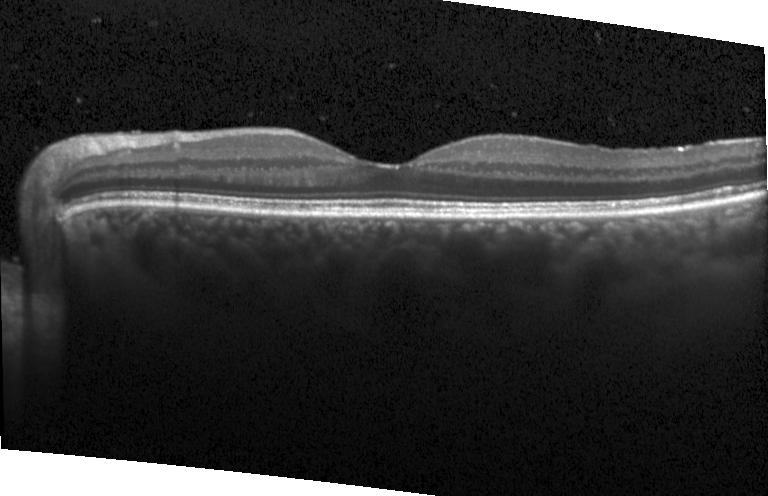

Macular OCT demonstrating no choroidal neovascularization, no diabetic macular edema, and no drusen.